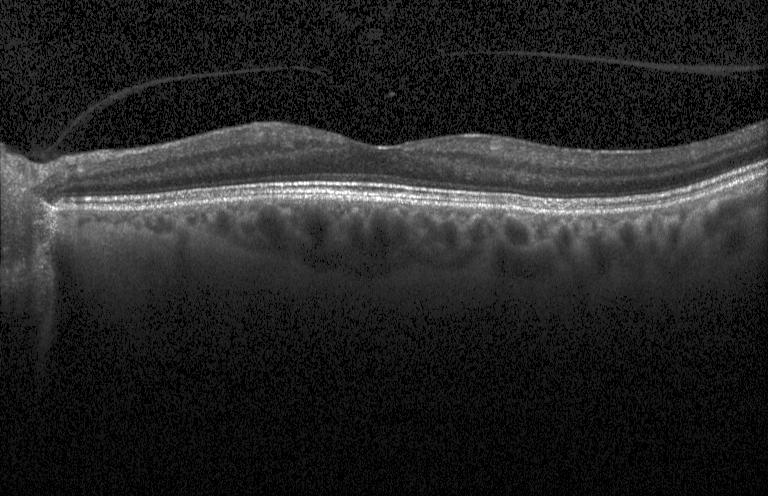

Optical coherence tomography scan. Heidelberg Spectralis OCT system. Diagnosis: no choroidal neovascularization, diabetic macular edema, or drusen.